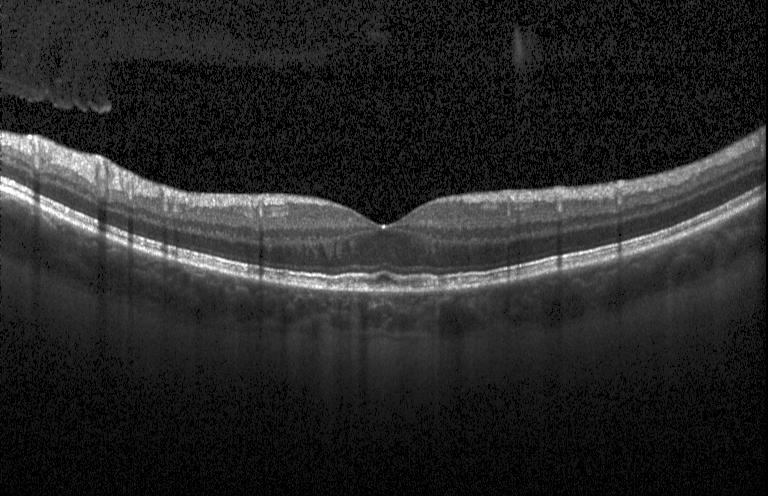
Impression: sub-RPE drusenoid deposits.